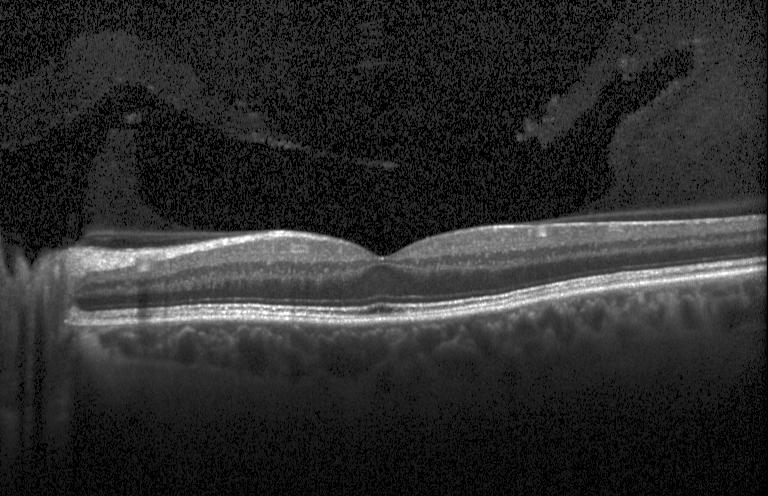

Centered on the fovea · OCT line scan.
This B-scan demonstrates no evidence of choroidal neovascularization, diabetic macular edema, or drusen.